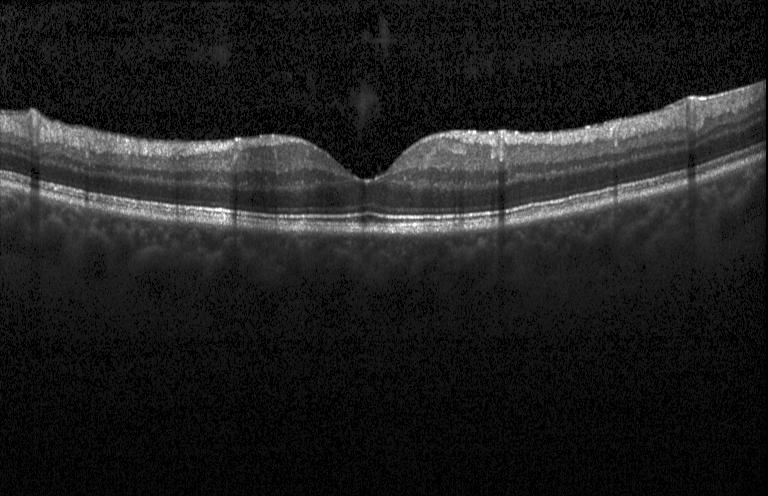
SD-OCT, optical coherence tomography B-scan
Diagnosis: no evidence of CNV, DME, or drusen.